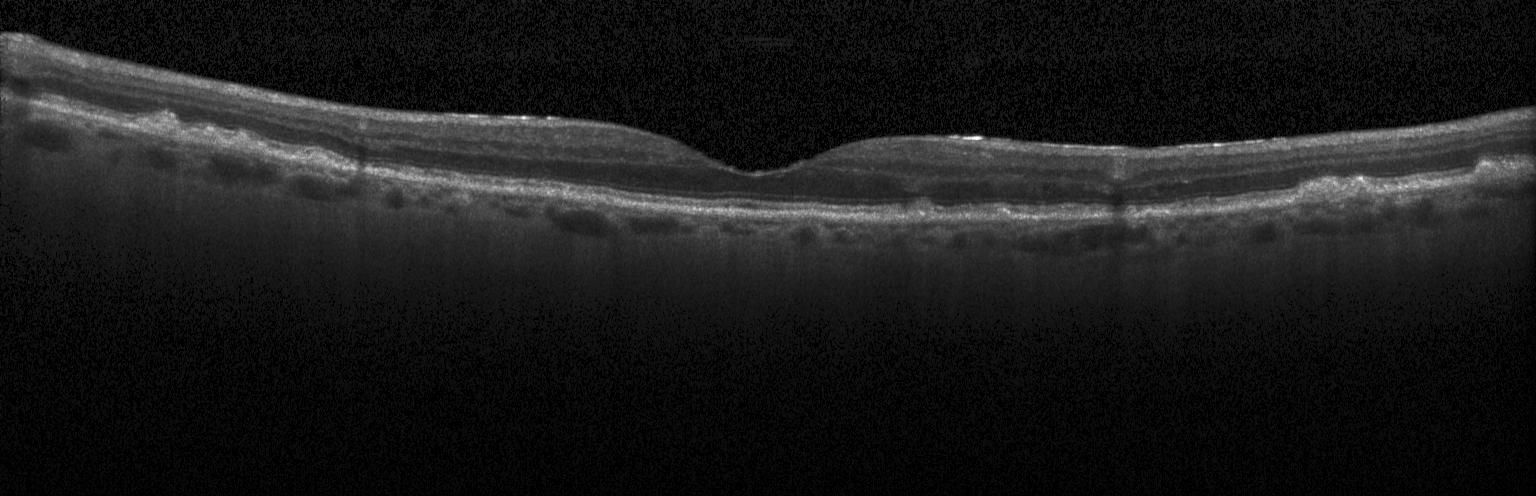 Retinal OCT cross-section showing drusen.